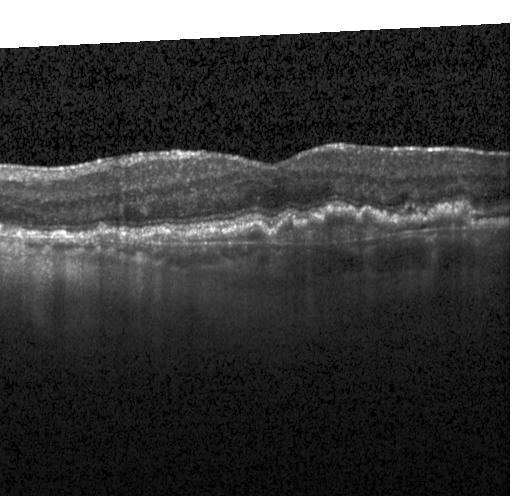 Spectral-domain OCT, optical coherence tomography B-scan, acquired on a Heidelberg Spectralis
Dx: choroidal neovascularization.